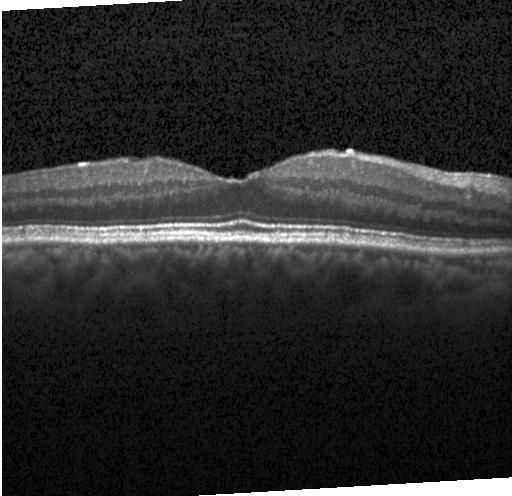

The scan shows no CNV, DME, or drusen.